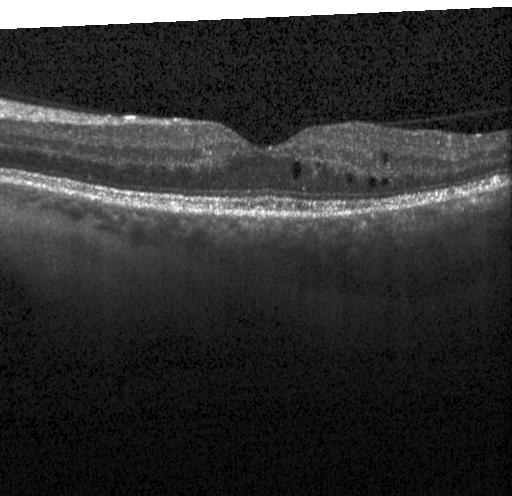

Dx: diabetic macular edema.